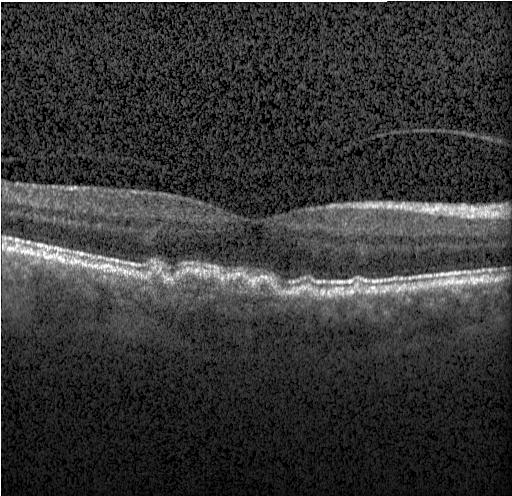
Finding: sub-RPE drusenoid deposits.